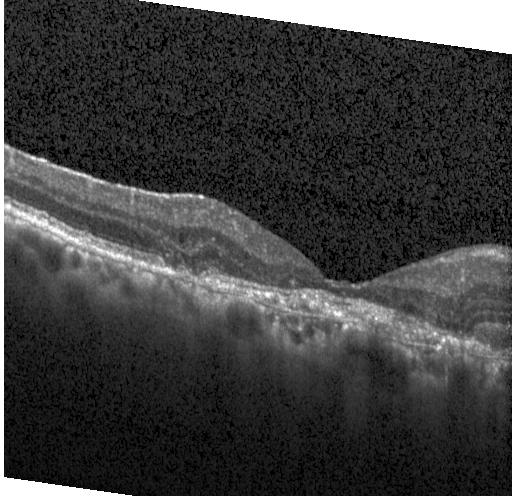 Fovea-centered; Heidelberg Spectralis OCT system; optical coherence tomography scan; SD-OCT. Impression: CNV.